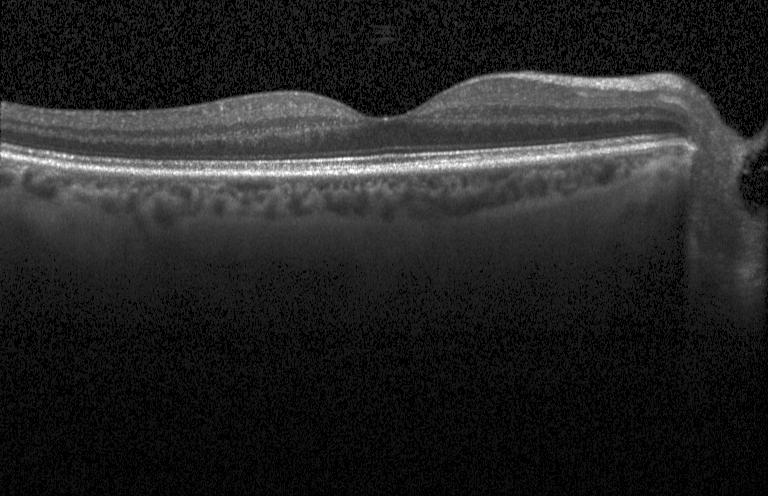 Acquired on a Heidelberg Spectralis; spectral-domain optical coherence tomography; fovea-centered; OCT line scan.
This B-scan demonstrates no evidence of choroidal neovascularization, diabetic macular edema, or drusen.